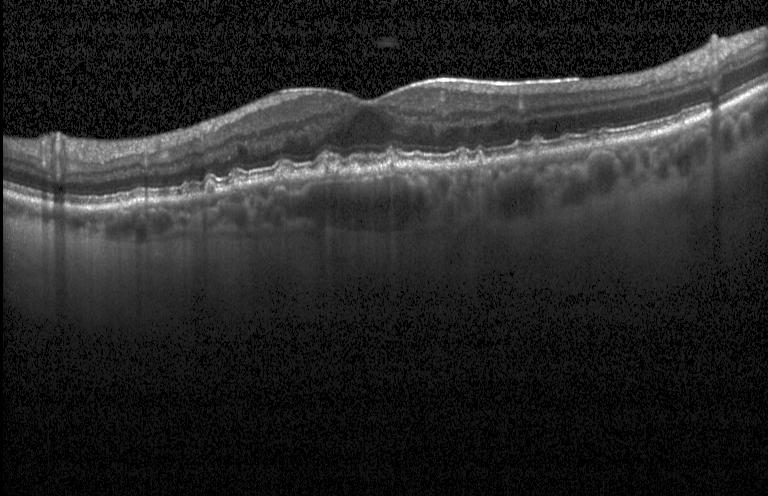
Macular OCT: sub-RPE drusenoid deposits.